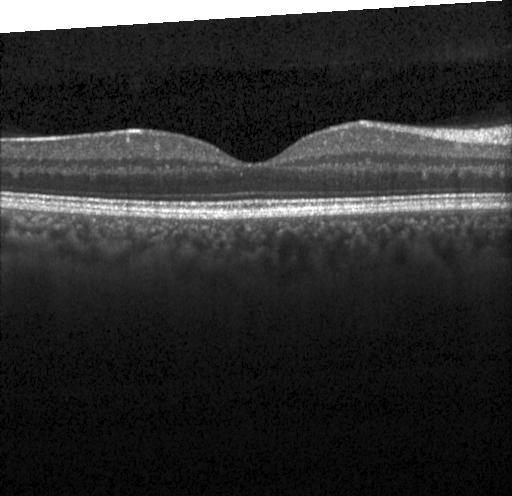 The scan shows no evidence of choroidal neovascularization, diabetic macular edema, or drusen.